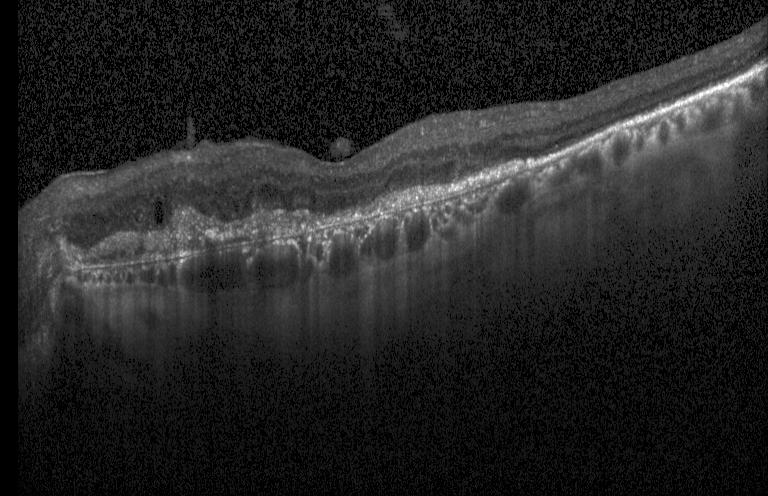 Retinal OCT cross-section
The scan shows a choroidal neovascular membrane.